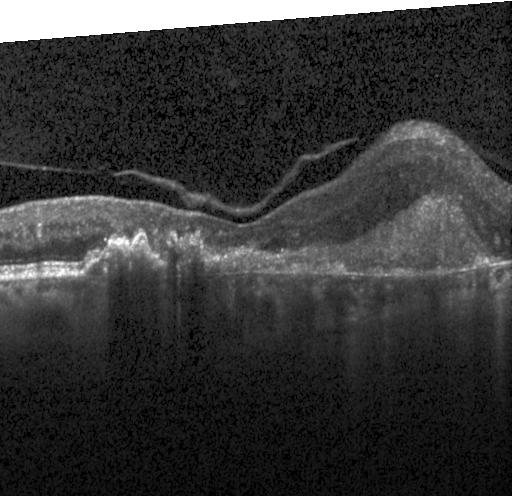

Retinal OCT cross-section — CNV.